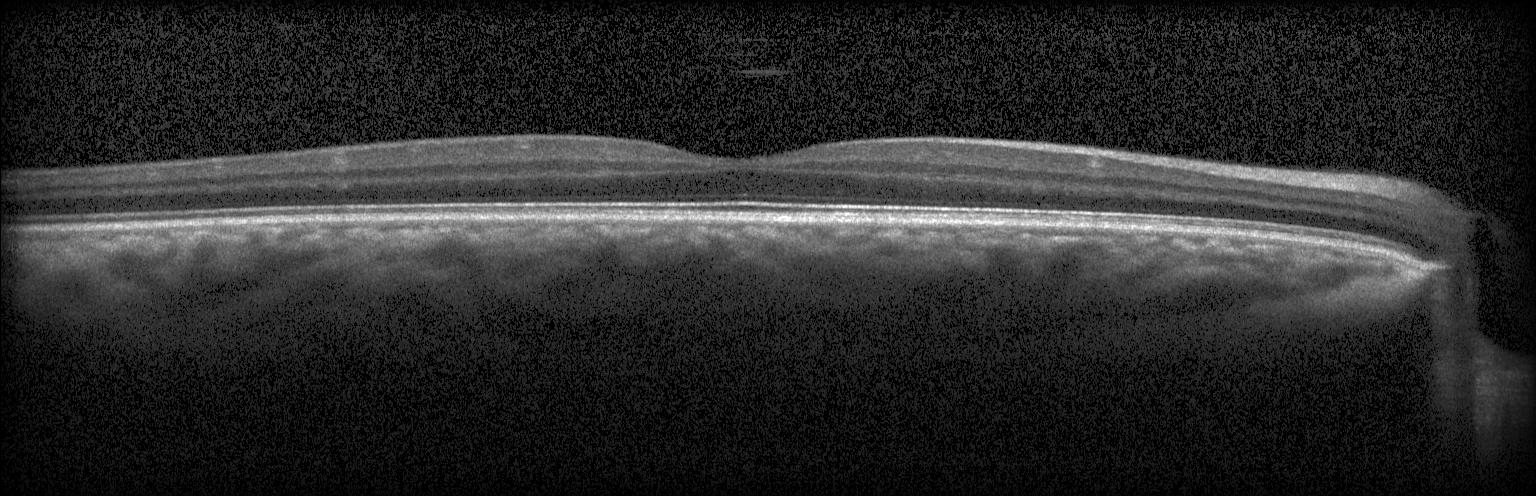 Diagnosis: neither choroidal neovascularization, diabetic macular edema, nor drusen.